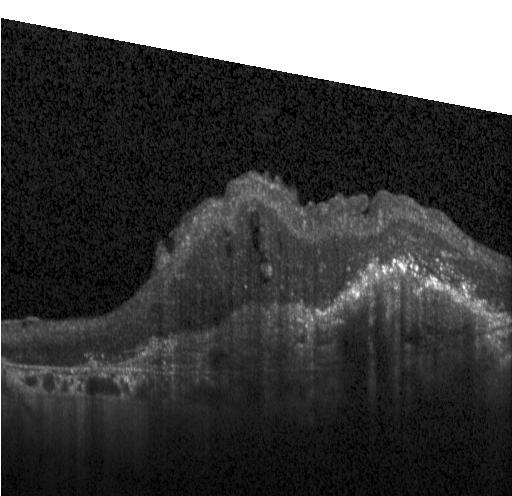 Horizontal scan through the fovea. Optical coherence tomography B-scan. SD-OCT
Impression: a choroidal neovascular membrane.